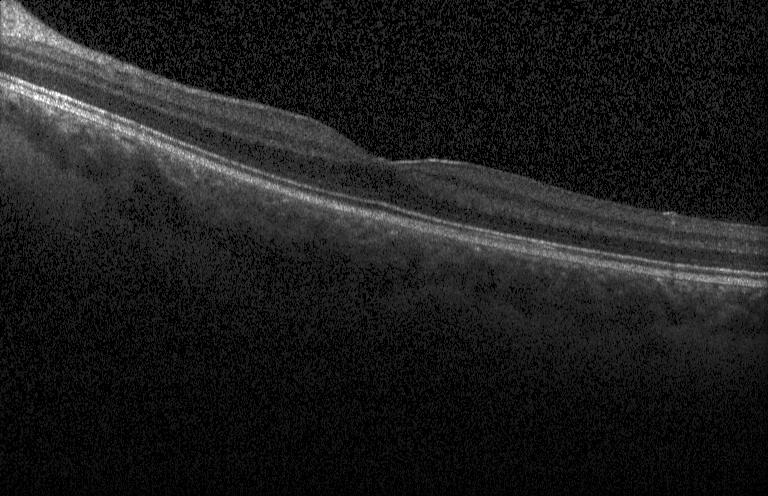

Horizontal scan through the fovea, retinal OCT B-scan, spectral-domain optical coherence tomography, instrument: Heidelberg Spectralis. Dx: neither choroidal neovascularization, diabetic macular edema, nor drusen.